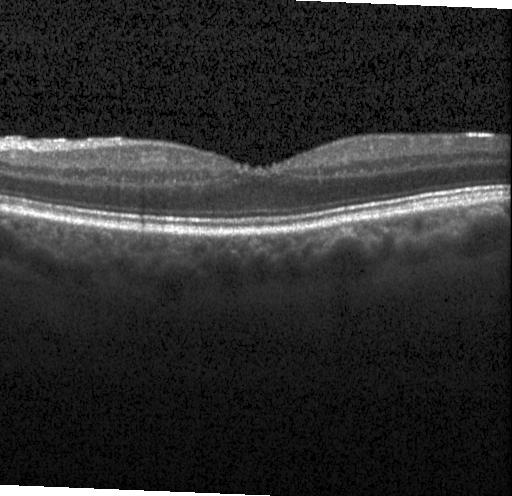
OCT line scan. Finding: neither CNV, DME, nor drusen.